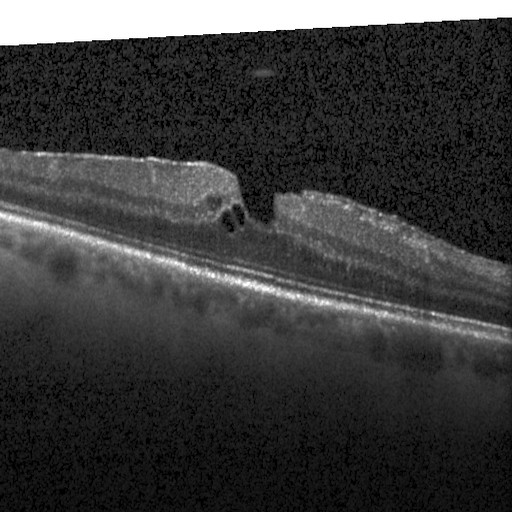
Optical coherence tomography B-scan. Heidelberg Spectralis. Spectral-domain optical coherence tomography. Fovea-centered. Macular OCT: DME.